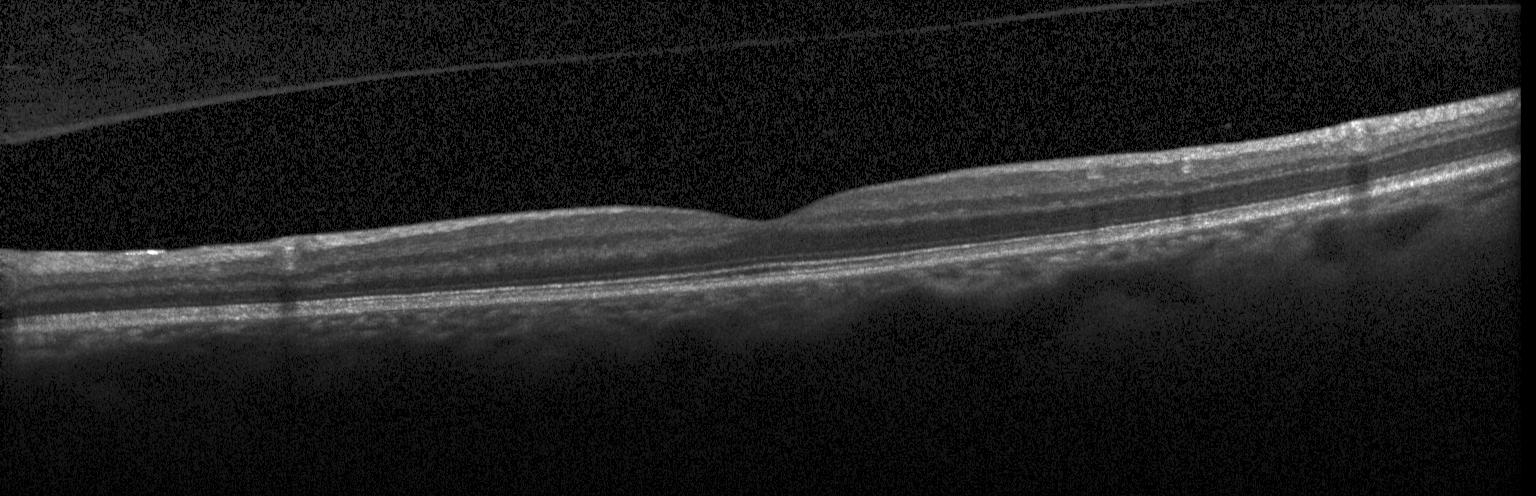

SD-OCT; optical coherence tomography scan.
Diagnosis: neither CNV, DME, nor drusen.